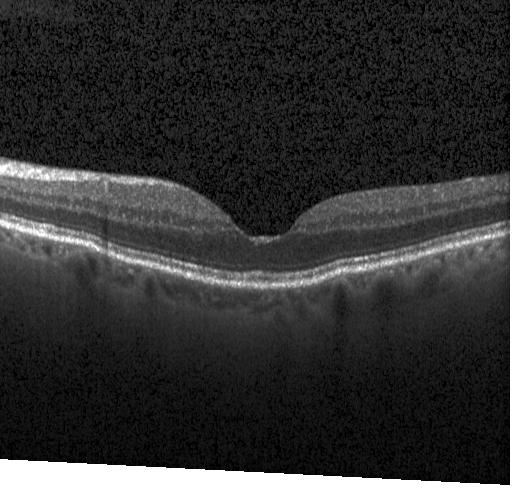 Impression: no evidence of CNV, DME, or drusen.